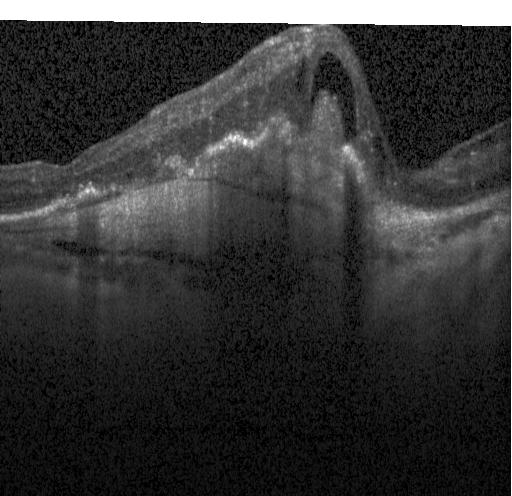

Diagnosis: a choroidal neovascular membrane.